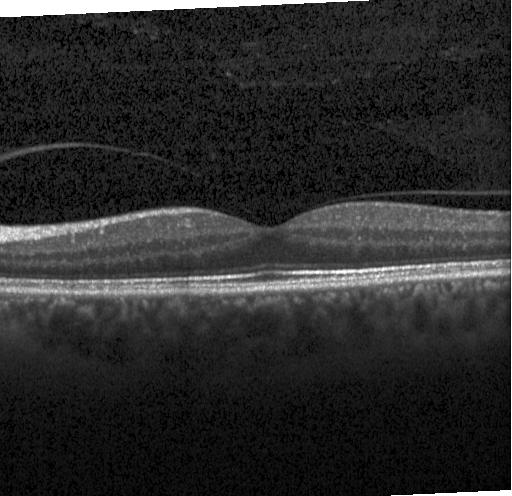 Diagnosis: no choroidal neovascularization, no diabetic macular edema, and no drusen.